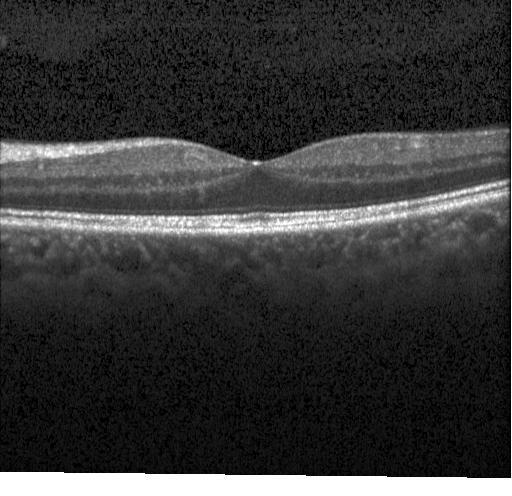

Impression: no evidence of choroidal neovascularization, diabetic macular edema, or drusen.